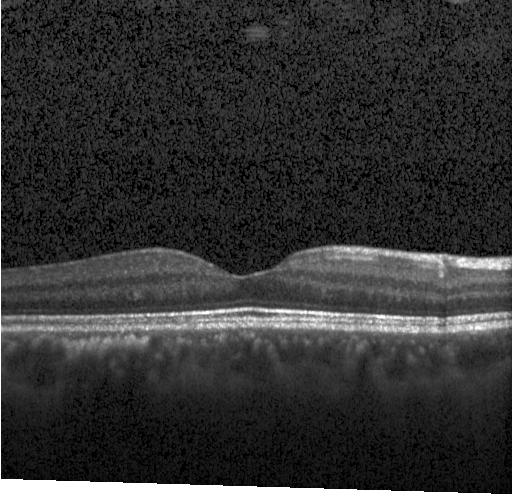

Diagnosis: no evidence of CNV, DME, or drusen.